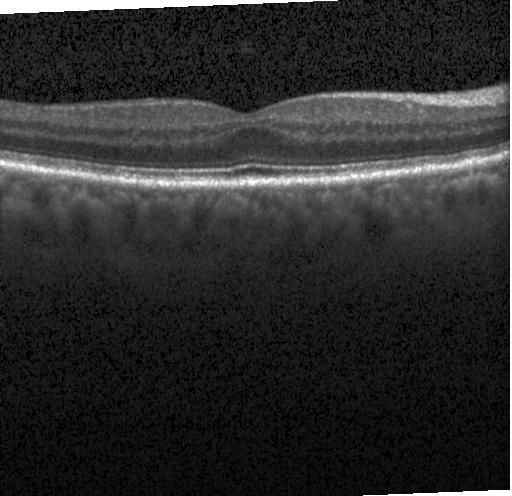 OCT finding: no choroidal neovascularization, no diabetic macular edema, and no drusen.